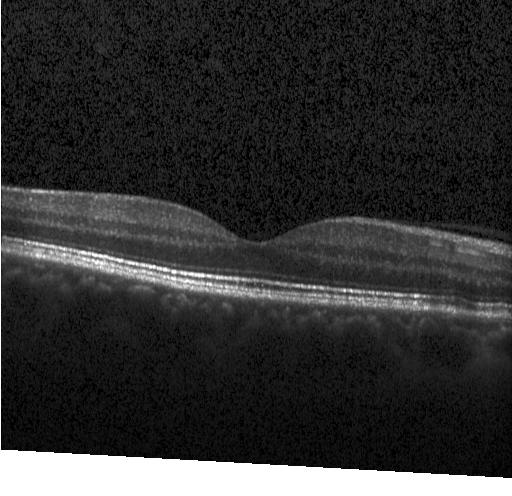

OCT B-scan.
Finding: no choroidal neovascularization, diabetic macular edema, or drusen.